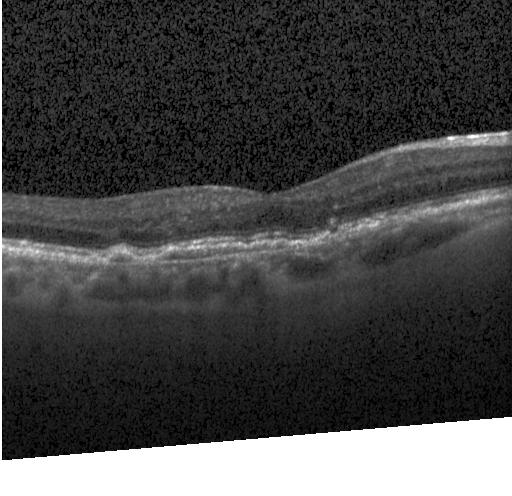

Spectral-domain optical coherence tomography · horizontal scan through the fovea · optical coherence tomography B-scan
Dx: choroidal neovascularization.